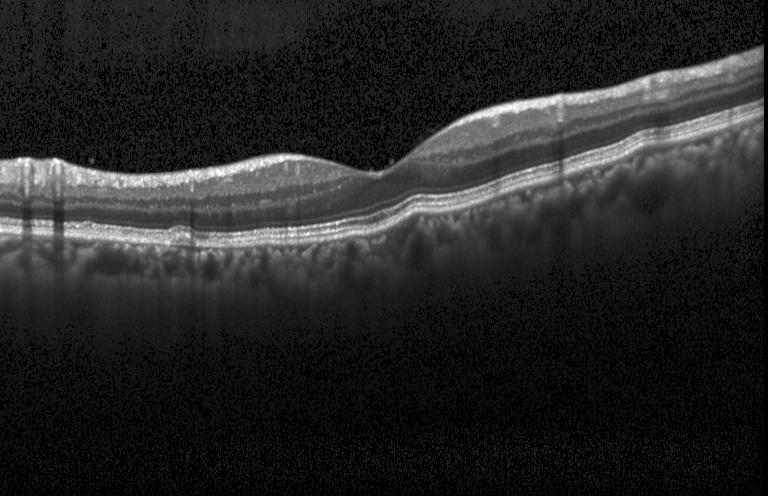

OCT line scan — Assessment: multiple drusen.